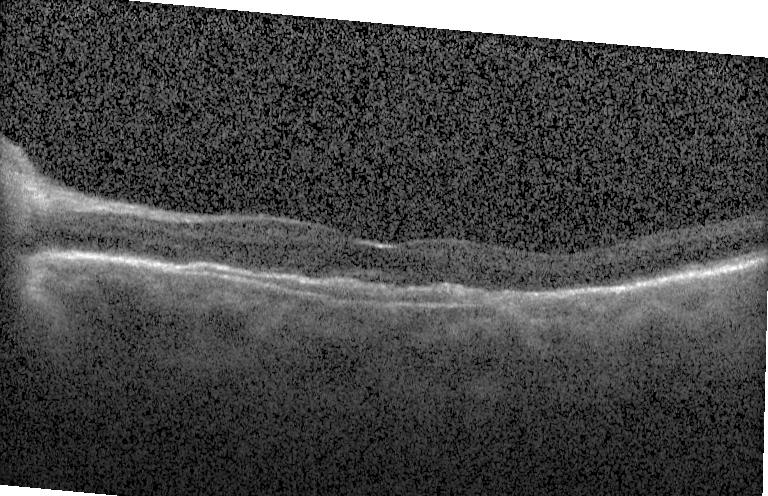

Diagnosis: a choroidal neovascular membrane.